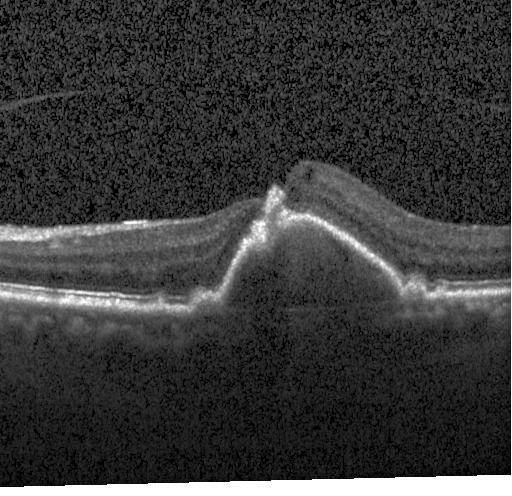

Through the macula. Retinal OCT B-scan. Instrument: Heidelberg Spectralis — Diagnosis: CNV.